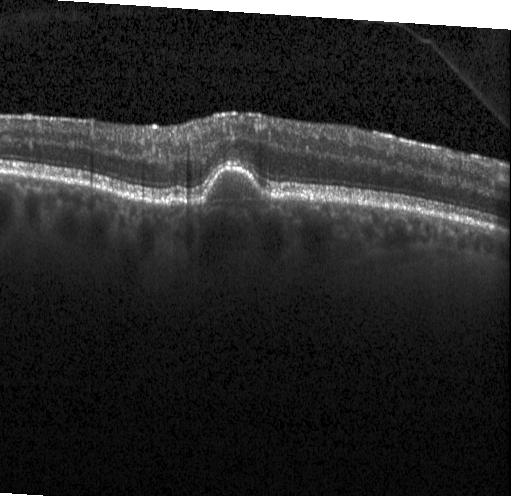

Finding: CNV.